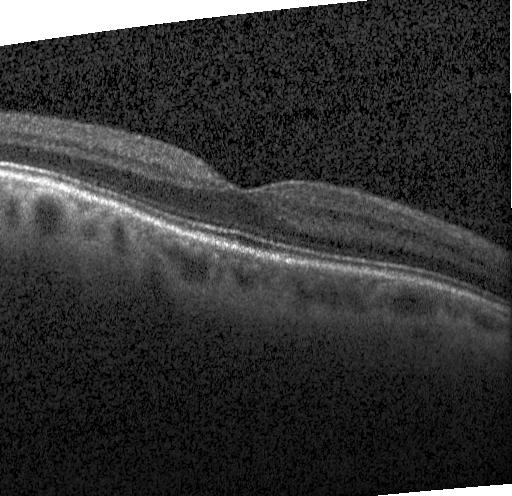

Instrument: Heidelberg Spectralis · horizontal scan through the fovea · OCT B-scan · spectral-domain OCT. Neither choroidal neovascularization, diabetic macular edema, nor drusen.